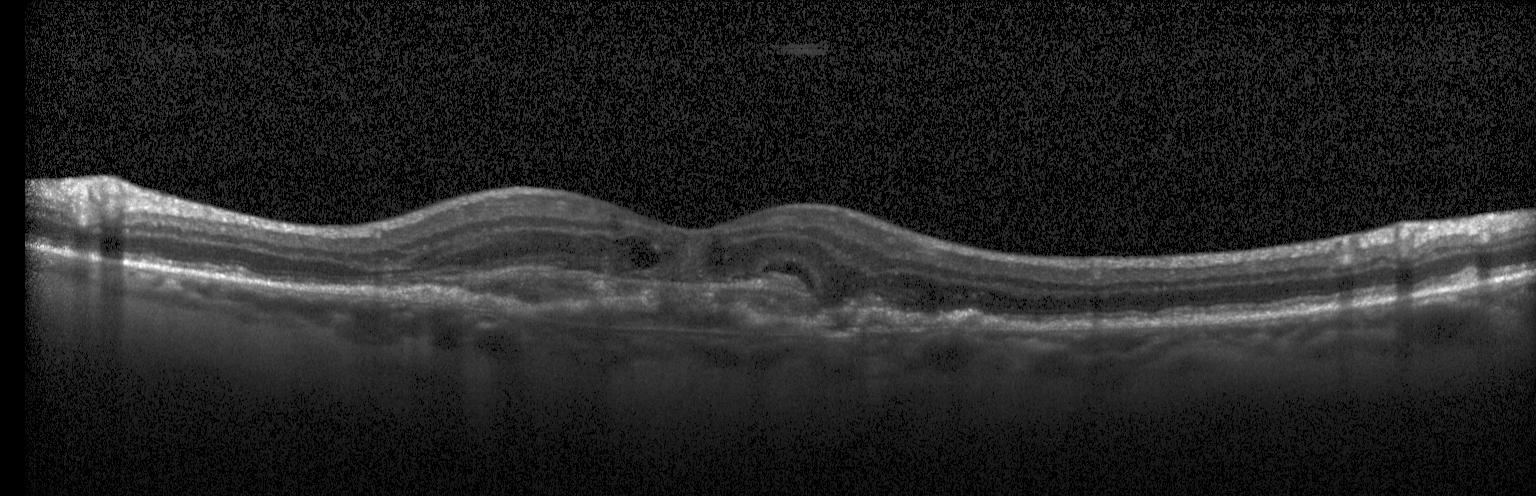
Retinal OCT B-scan. Horizontal scan through the fovea. Assessment: CNV.